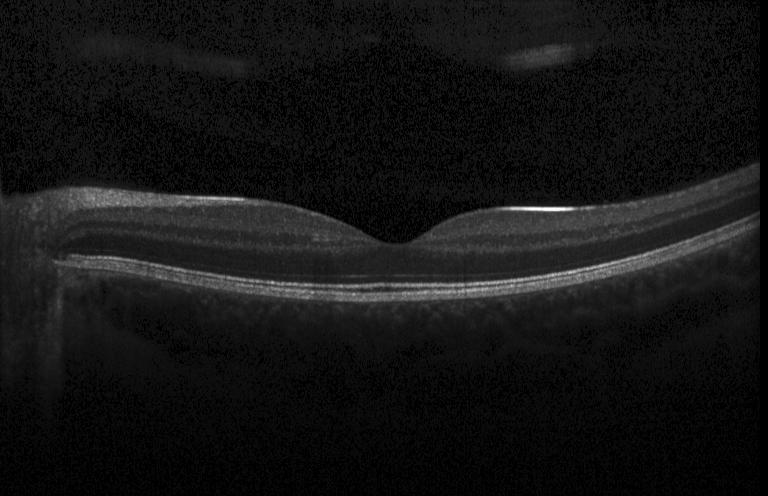 Spectral-domain optical coherence tomography; through the macula; retinal OCT B-scan.
Diagnosis: no evidence of choroidal neovascularization, diabetic macular edema, or drusen.